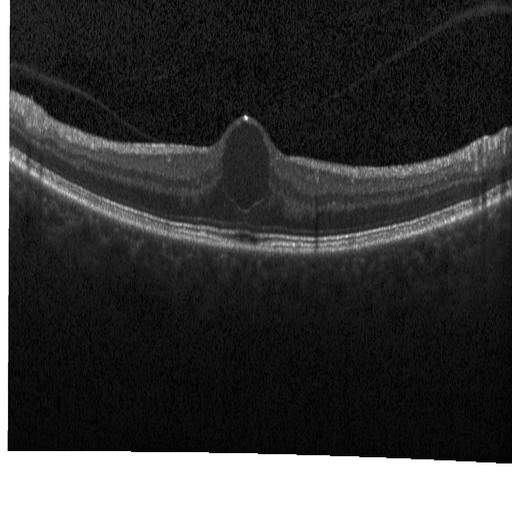 Retinal OCT cross-section. Finding: diabetic macular edema (DME).